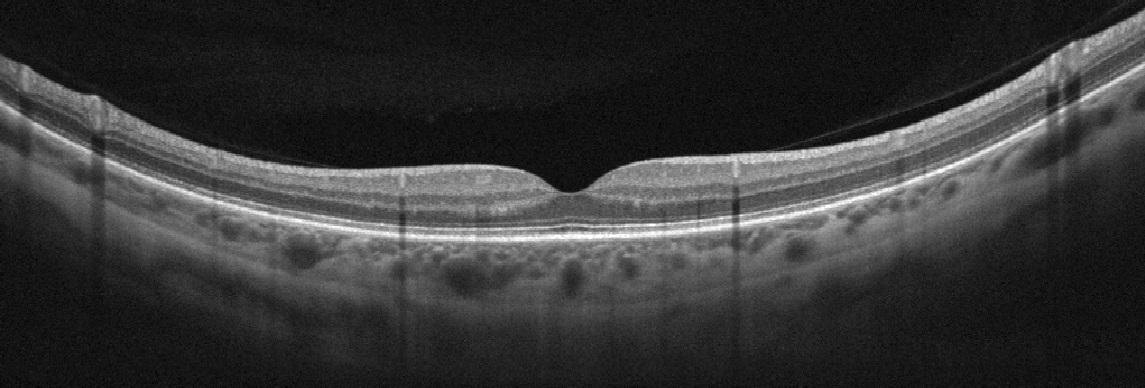 OCT B-scan · Optovue Avanti RTVue XR · fovea-centered
The scan shows no evidence of AMD, DME, ERM, RAO, RVO, or VID.